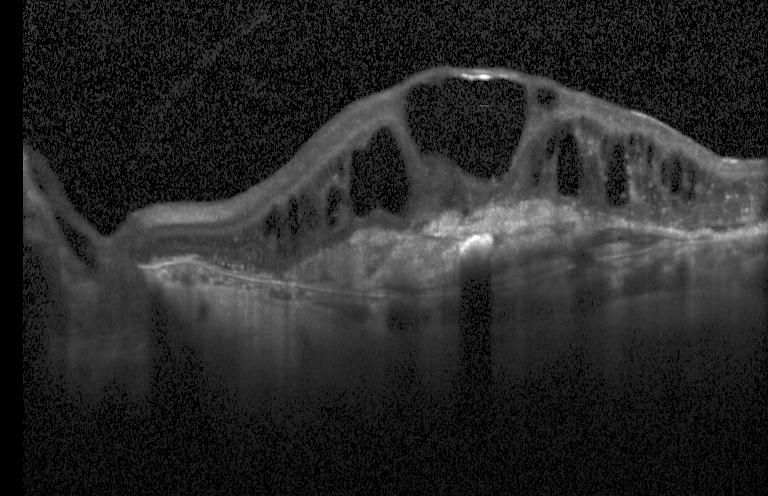 OCT line scan. The scan shows choroidal neovascularization (CNV).